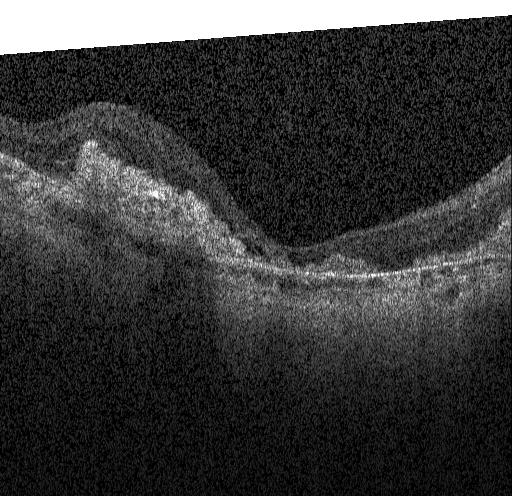 Retinal OCT B-scan — Finding: a choroidal neovascular membrane.